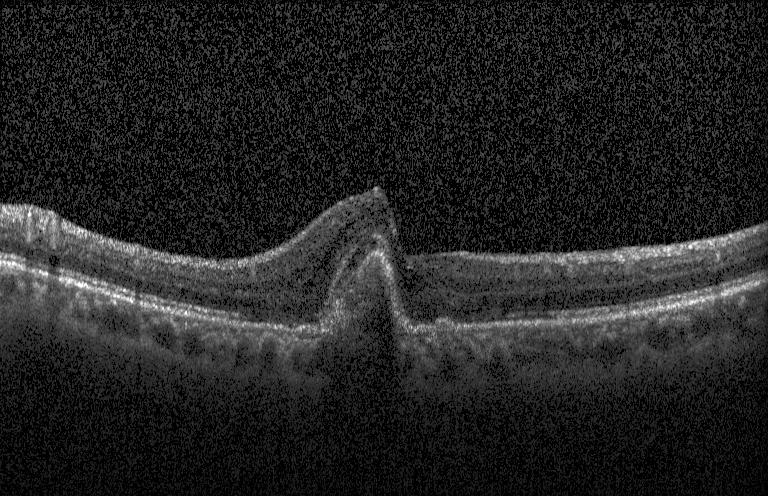
Retinal OCT B-scan; instrument: Heidelberg Spectralis; SD-OCT; fovea-centered.
Finding: a choroidal neovascular membrane.